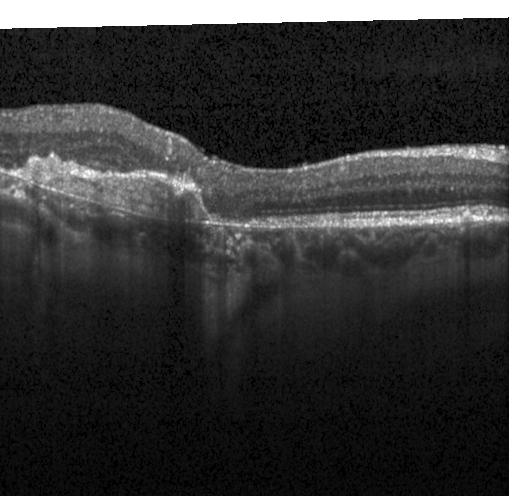

Acquired on a Heidelberg Spectralis. Spectral-domain OCT. Optical coherence tomography scan. Centered on the fovea. Finding: CNV.